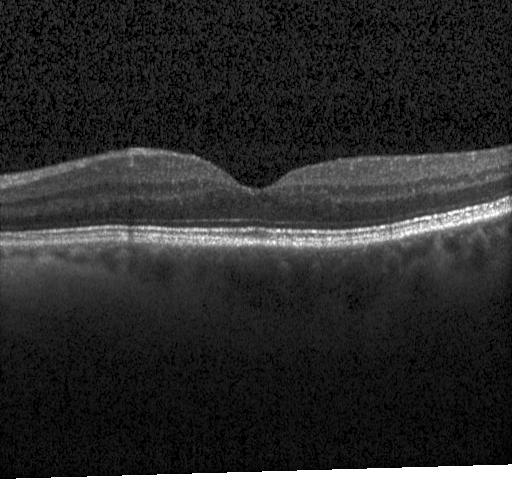 Retinal OCT cross-section — Finding: neither CNV, DME, nor drusen.